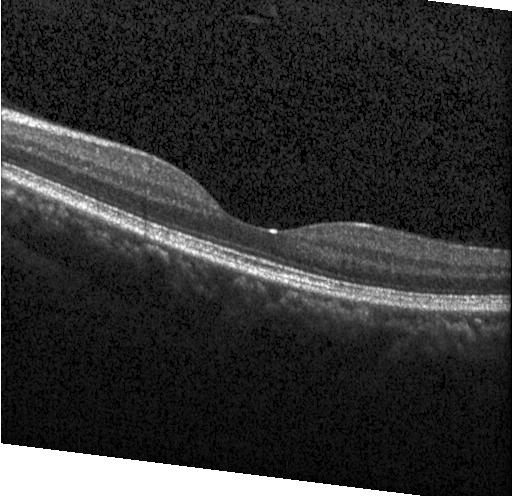

OCT finding: no choroidal neovascularization, no diabetic macular edema, and no drusen.